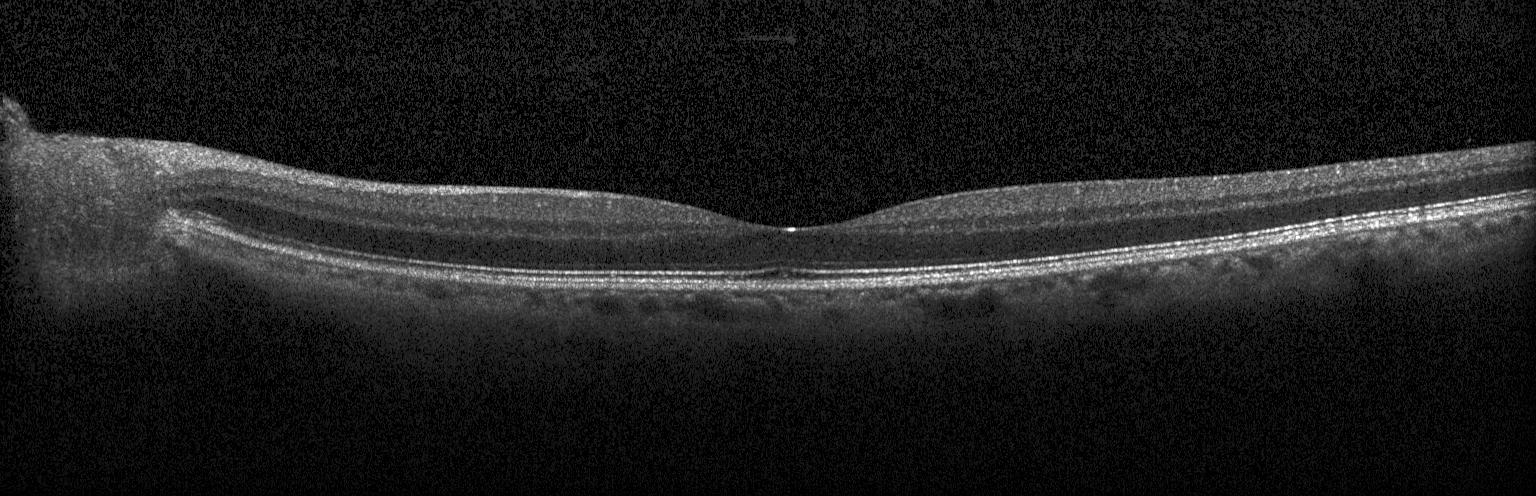
Horizontal scan through the fovea · Heidelberg Spectralis OCT system · OCT B-scan — Neither choroidal neovascularization, diabetic macular edema, nor drusen.